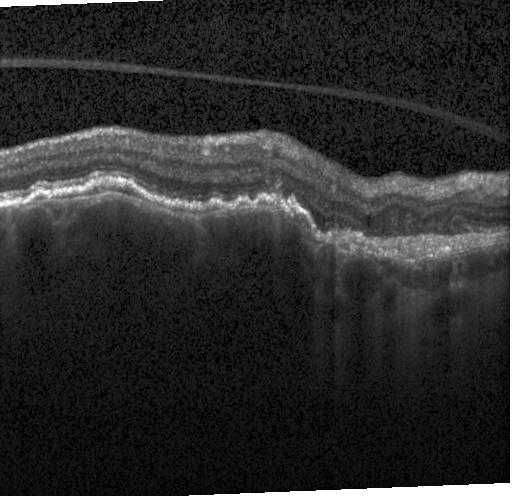

Impression: a choroidal neovascular membrane.